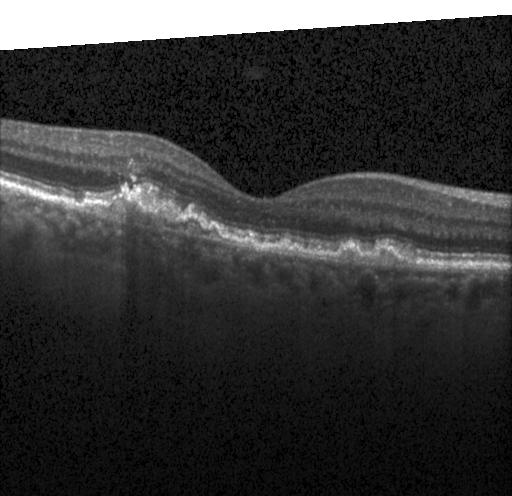 Diagnosis: CNV.